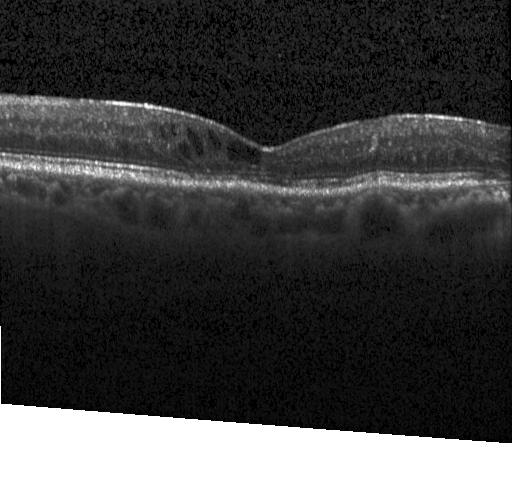

OCT B-scan; instrument: Heidelberg Spectralis — Impression: diabetic macular edema (DME).